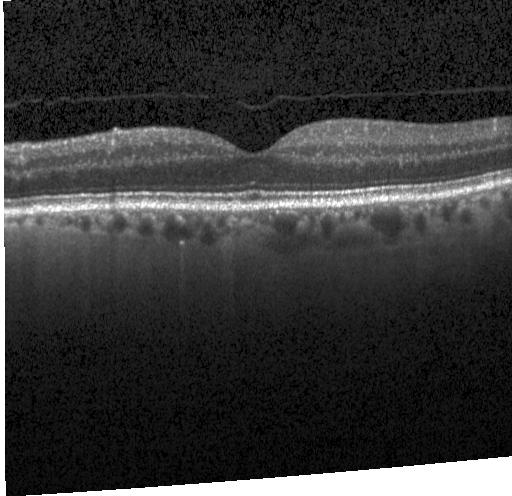 Impression: no evidence of CNV, DME, or drusen.